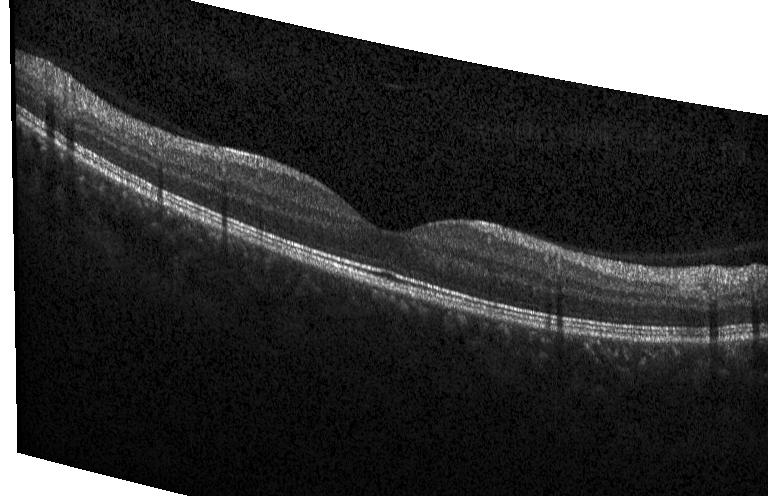

Impression: no evidence of CNV, DME, or drusen.